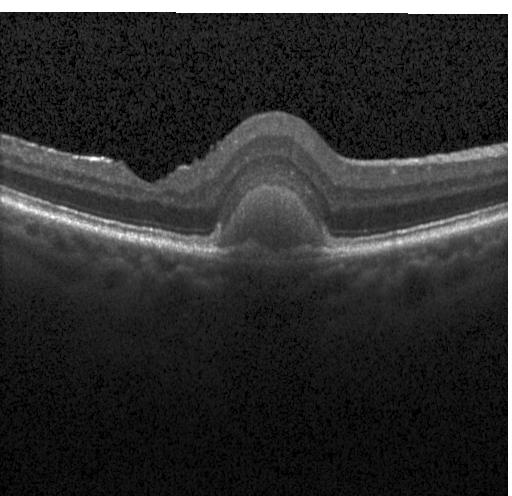

Optical coherence tomography B-scan.
Diagnosis: choroidal neovascularization (CNV).